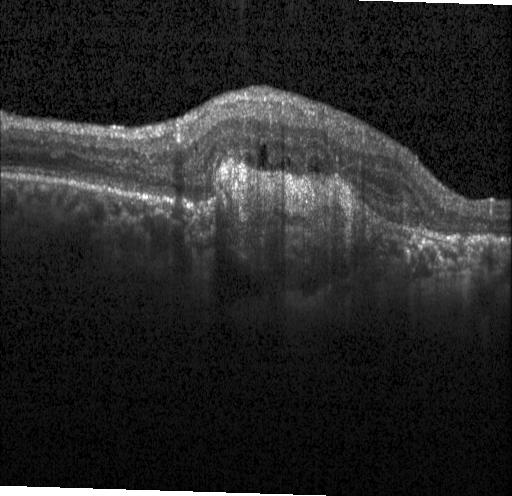

Optical coherence tomography B-scan
OCT finding: choroidal neovascularization.